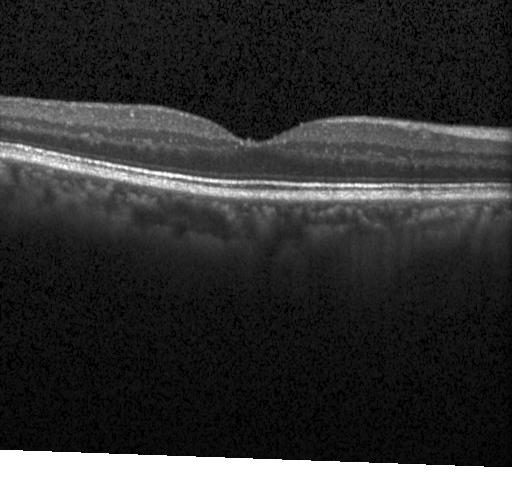 Acquired on a Heidelberg Spectralis. Macular scan. Retinal OCT cross-section
Dx: no CNV, no DME, and no drusen.